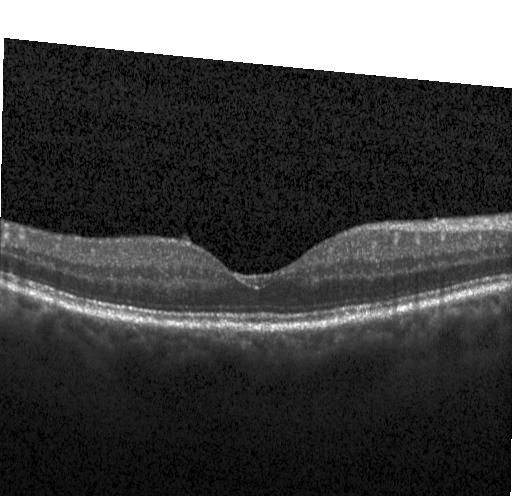 Fovea-centered; optical coherence tomography scan
The scan shows no evidence of choroidal neovascularization, diabetic macular edema, or drusen.